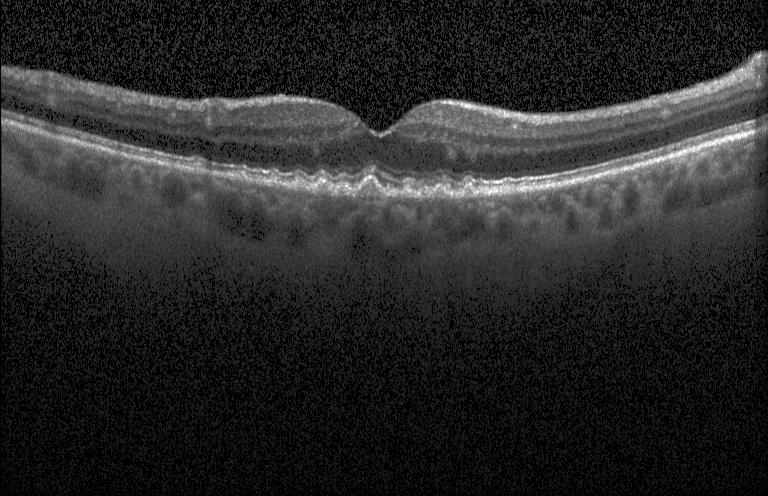 OCT scan showing drusen.